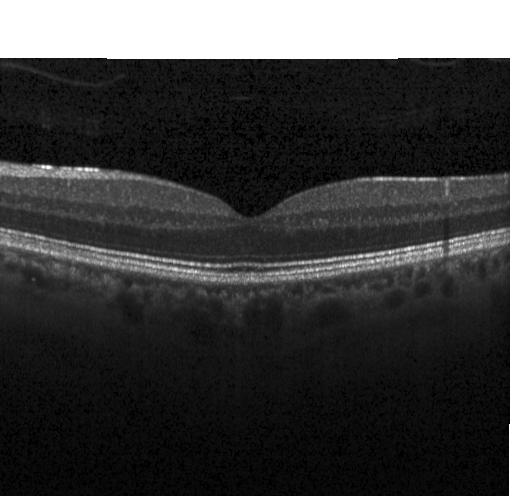 Diagnosis: no choroidal neovascularization, diabetic macular edema, or drusen.